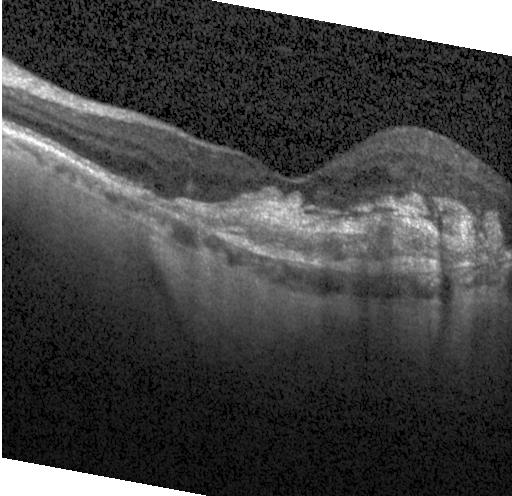 Spectral-domain OCT, OCT line scan, acquired on a Heidelberg Spectralis
Dx: CNV.